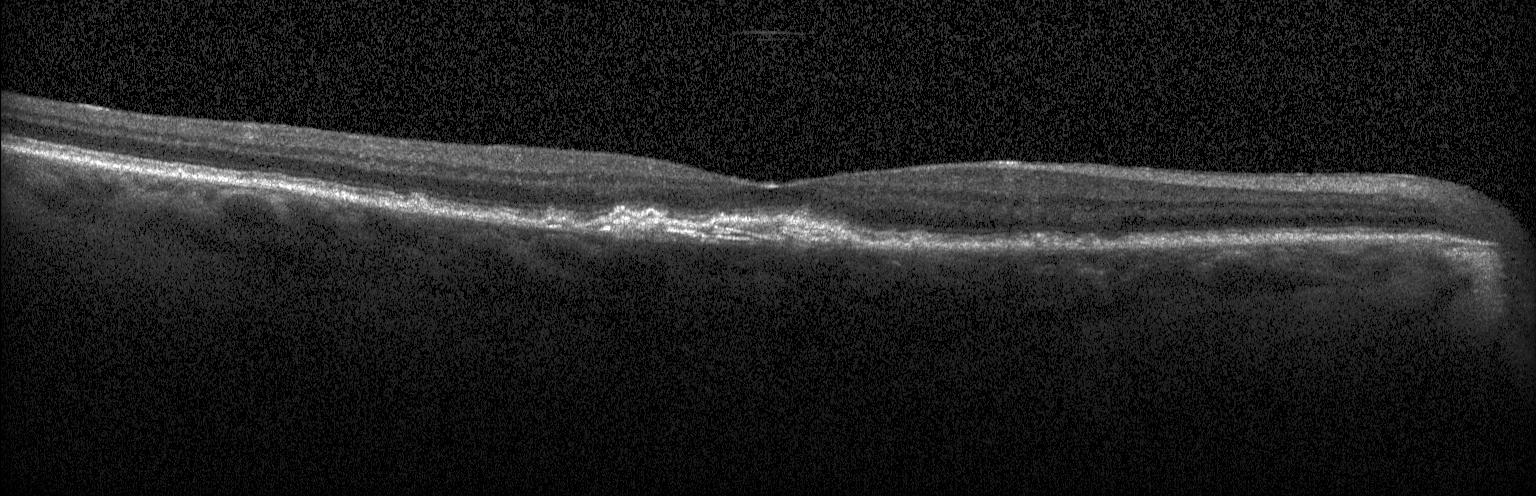 Through the macula; retinal OCT cross-section; Heidelberg Spectralis. Dx: a choroidal neovascular membrane.